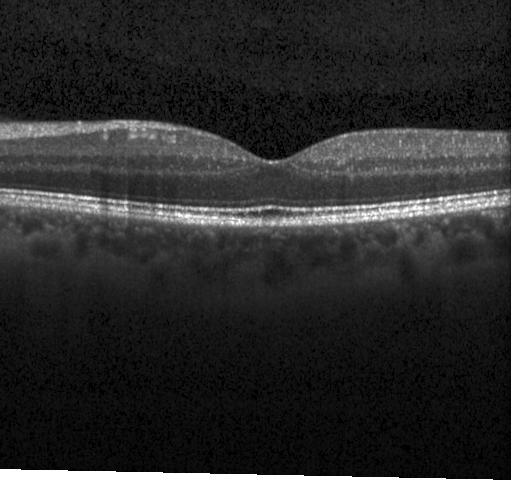 OCT B-scan · centered on the fovea.
Finding: no CNV, DME, or drusen.